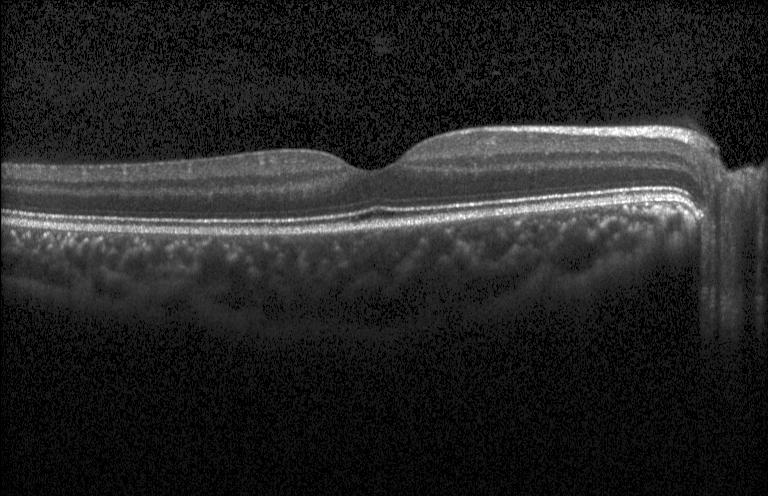
Impression: no CNV, no DME, and no drusen.